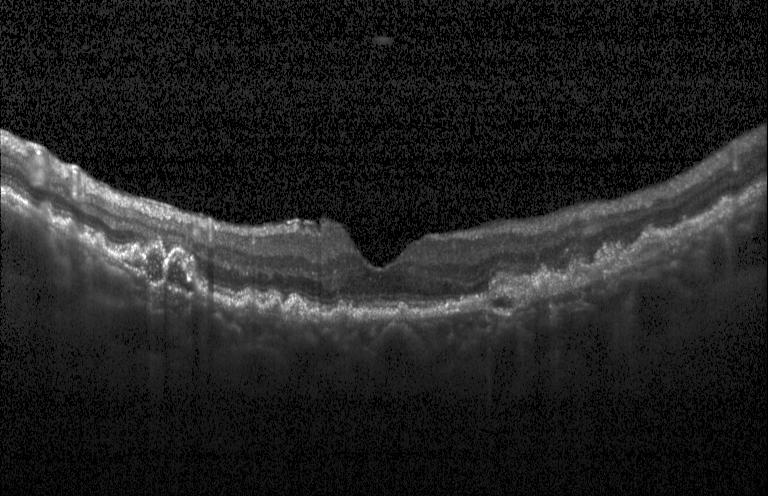

Retinal OCT cross-section showing a choroidal neovascular membrane.